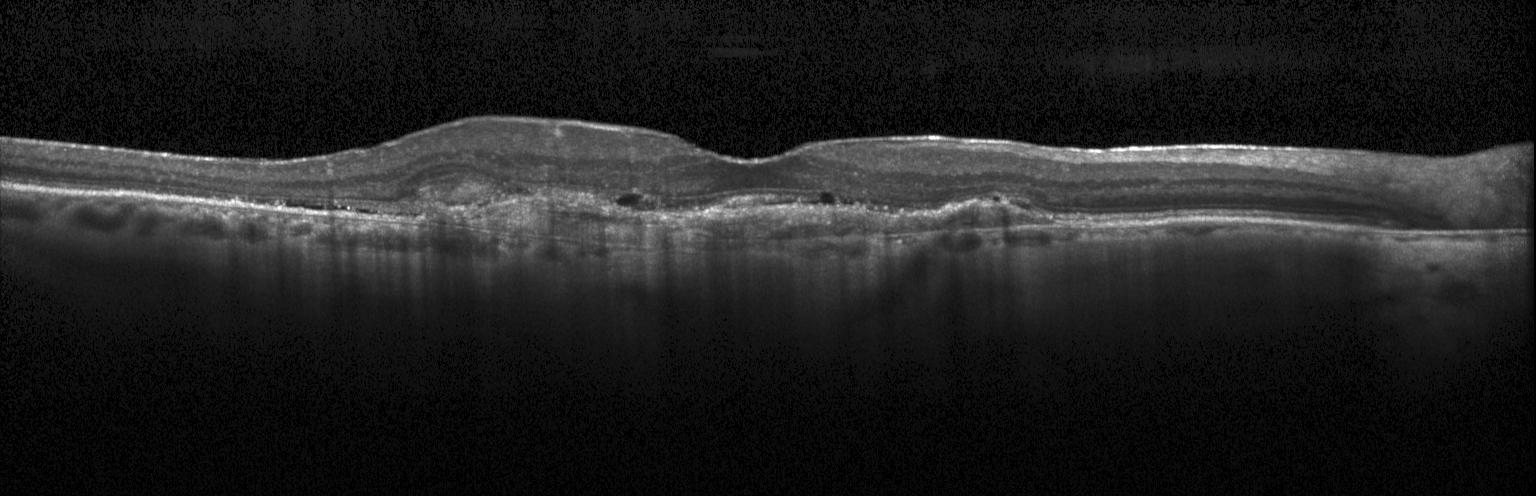

OCT scan showing a choroidal neovascular membrane.